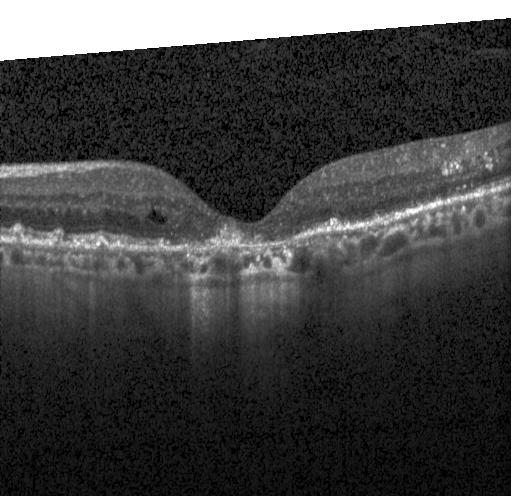

Heidelberg Spectralis OCT system; macular scan; optical coherence tomography scan; spectral-domain OCT. Dx: CNV.